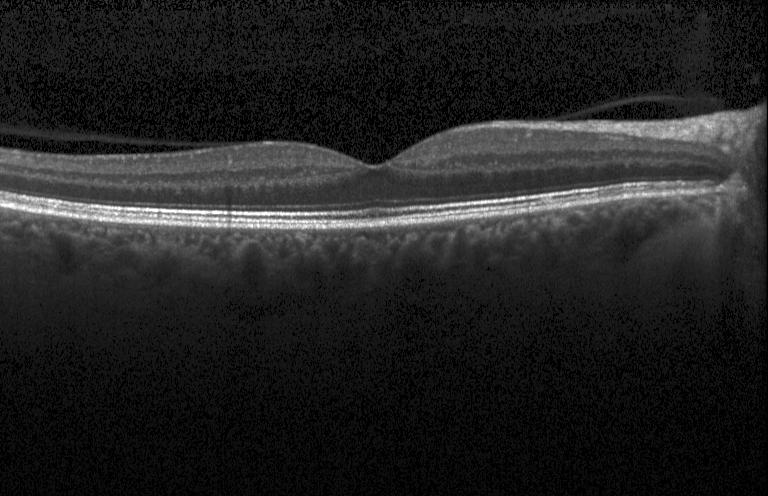 Spectral-domain OCT B-scan: no choroidal neovascularization, diabetic macular edema, or drusen.